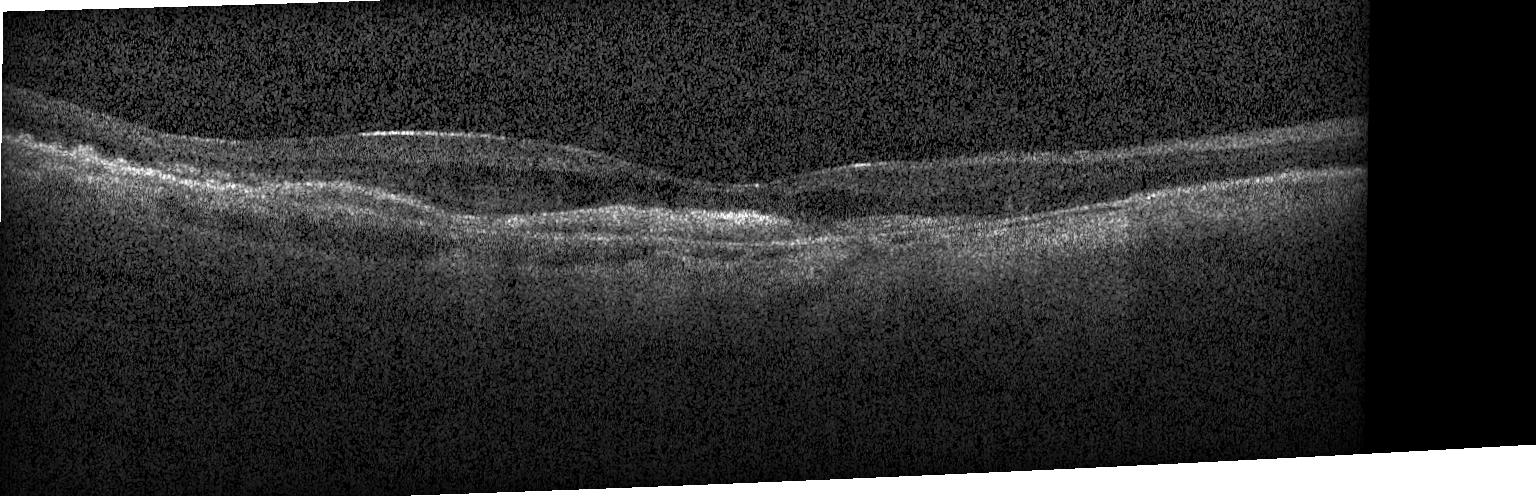
Optical coherence tomography scan
Impression: choroidal neovascularization.